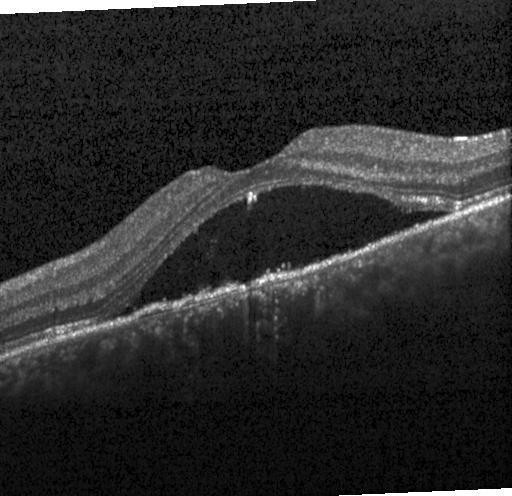

Spectral-domain optical coherence tomography; horizontal scan through the fovea; retinal OCT cross-section — This B-scan demonstrates CNV.